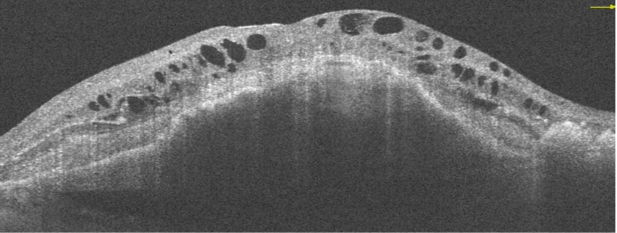

Retinal OCT cross-section · instrument: Optovue Avanti RTVue XR
Assessment: age-related macular degeneration.